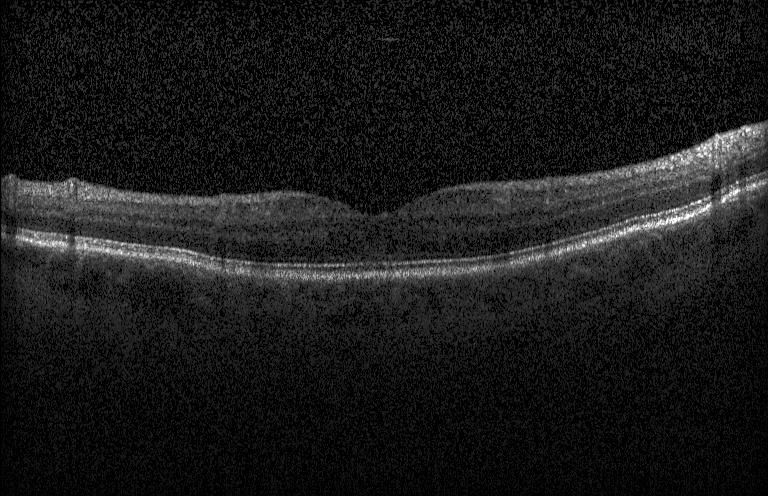
Retinal OCT B-scan. Acquired on a Heidelberg Spectralis.
Finding: no choroidal neovascularization, no diabetic macular edema, and no drusen.